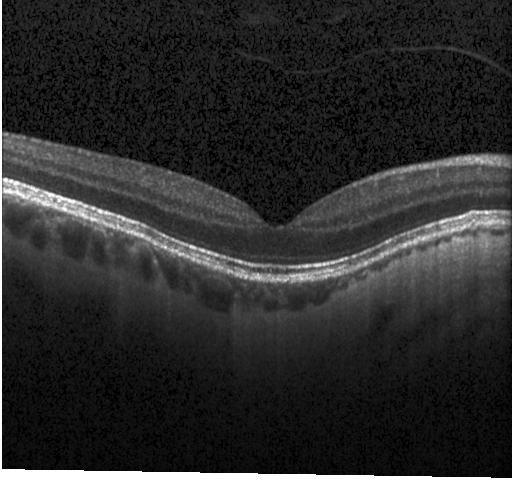
Spectral-domain OCT B-scan: no choroidal neovascularization, diabetic macular edema, or drusen.